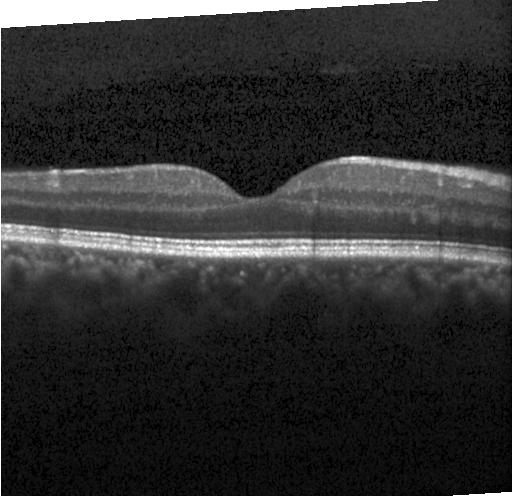 Retinal OCT B-scan; horizontal scan through the fovea; spectral-domain OCT. Diagnosis: no CNV, DME, or drusen.